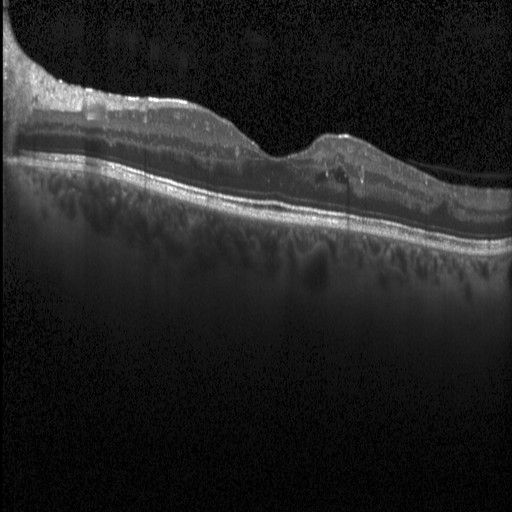

Retinal OCT B-scan. Heidelberg Spectralis OCT system. Through the macula — This B-scan demonstrates diabetic macular edema.